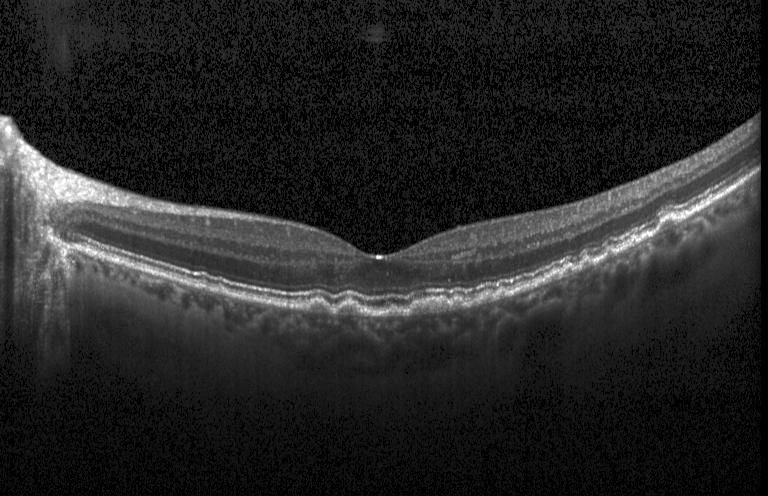

Instrument: Heidelberg Spectralis. OCT B-scan. Macular scan. SD-OCT — The scan shows sub-RPE drusenoid deposits.